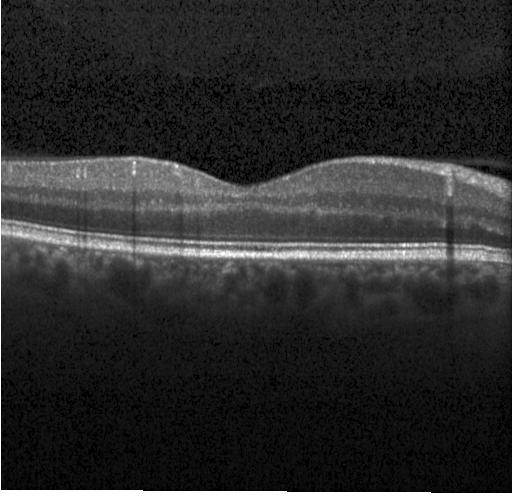
Retinal OCT cross-section, SD-OCT.
Assessment: no CNV, DME, or drusen.